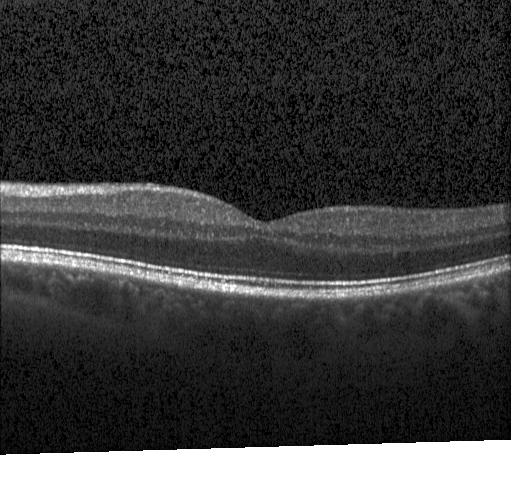
Retinal OCT cross-section — Diagnosis: no evidence of choroidal neovascularization, diabetic macular edema, or drusen.